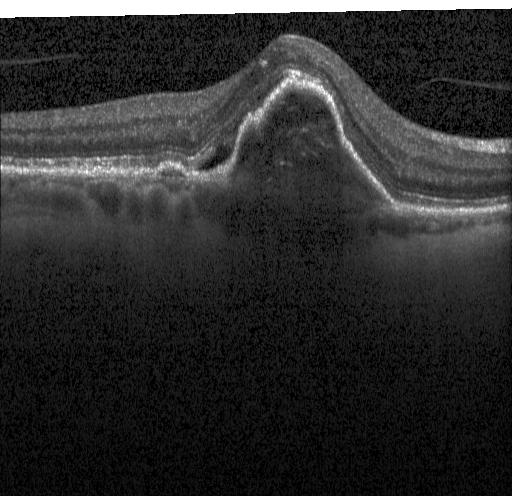

OCT scan showing a choroidal neovascular membrane.